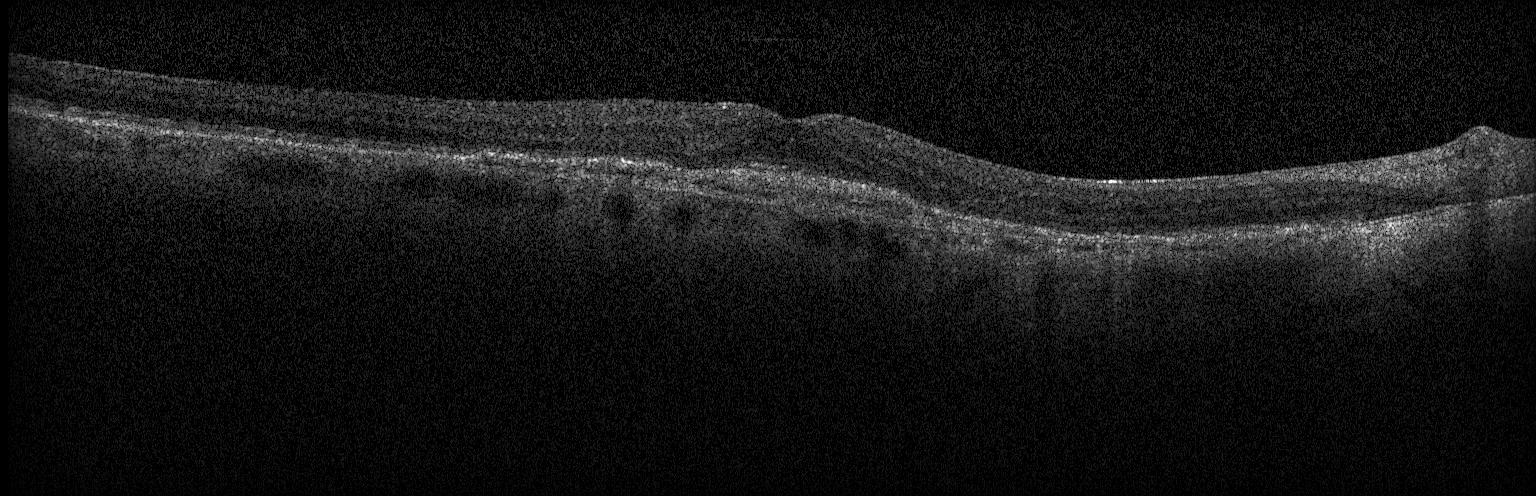

Spectral-domain optical coherence tomography · instrument: Heidelberg Spectralis · retinal OCT B-scan — OCT finding: a choroidal neovascular membrane.